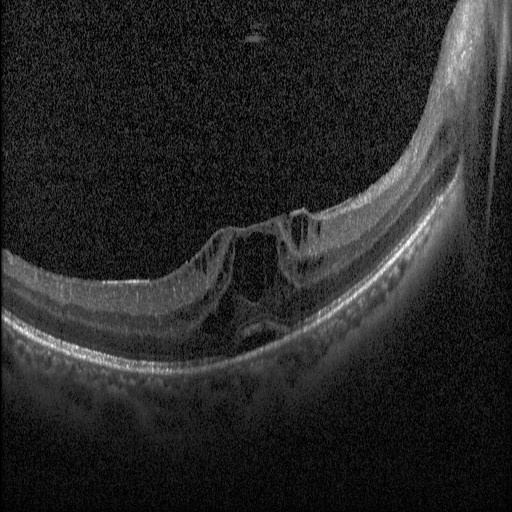

Retinal OCT cross-section. Impression: diabetic macular edema.